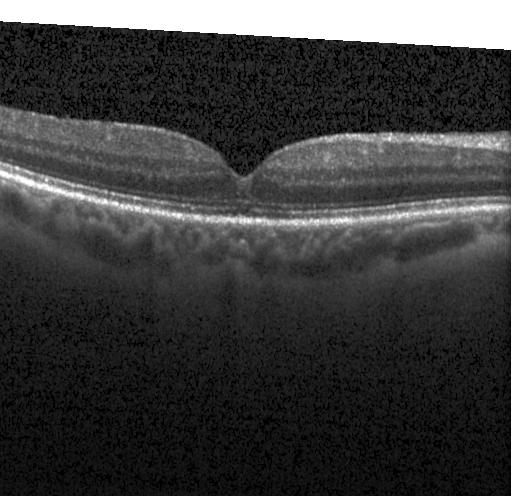 Macular OCT: no CNV, DME, or drusen.